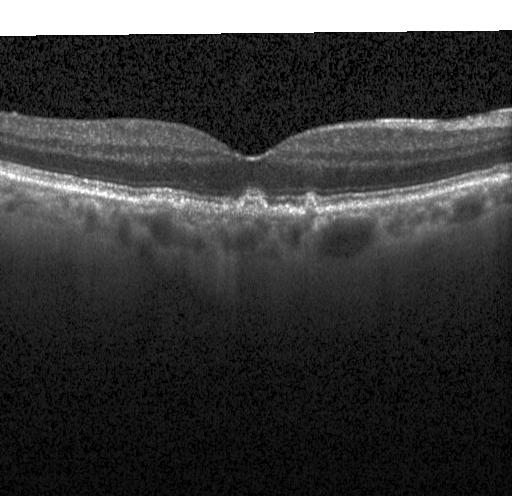
Diagnosis: sub-RPE drusenoid deposits.